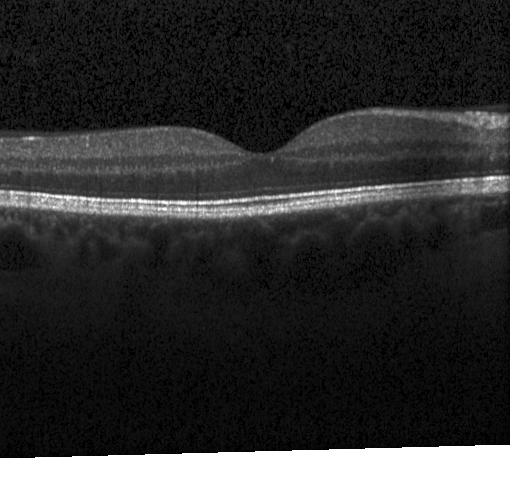

OCT B-scan showing no choroidal neovascularization, diabetic macular edema, or drusen.